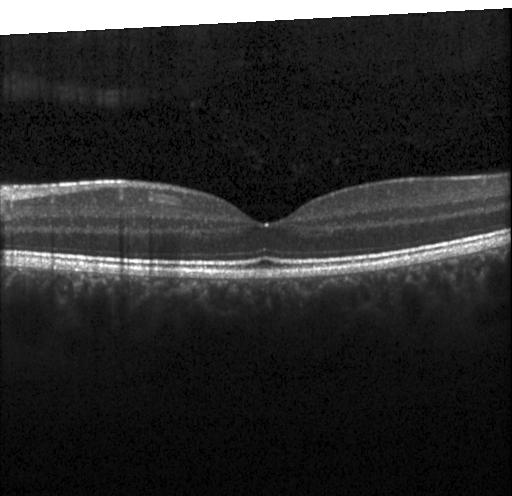
Retinal OCT B-scan; spectral-domain optical coherence tomography
Macular OCT: no choroidal neovascularization, no diabetic macular edema, and no drusen.